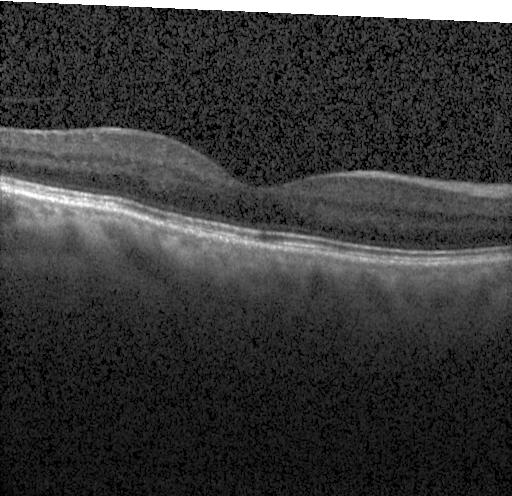
No CNV, no DME, and no drusen.